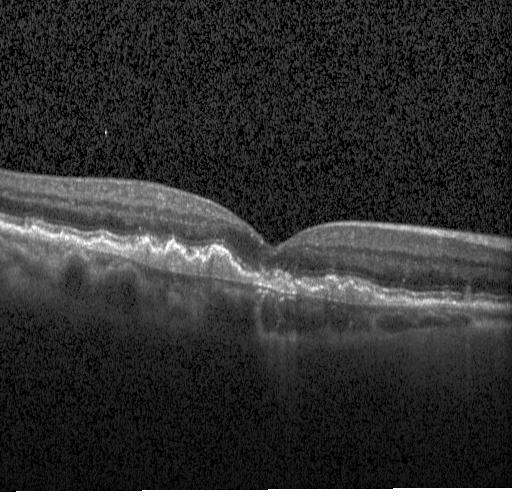

OCT B-scan; fovea-centered; spectral-domain optical coherence tomography. The scan shows choroidal neovascularization (CNV).